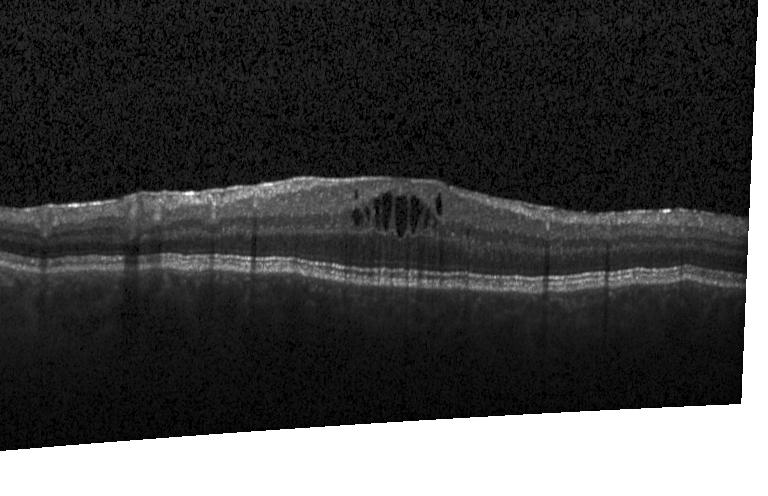

OCT line scan; SD-OCT. DME.